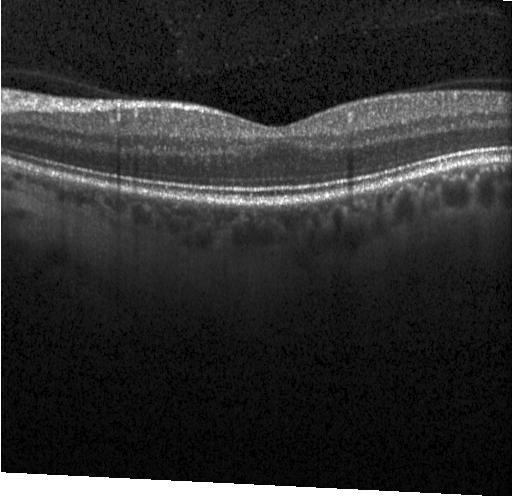

OCT B-scan · horizontal scan through the fovea
Impression: no CNV, no DME, and no drusen.